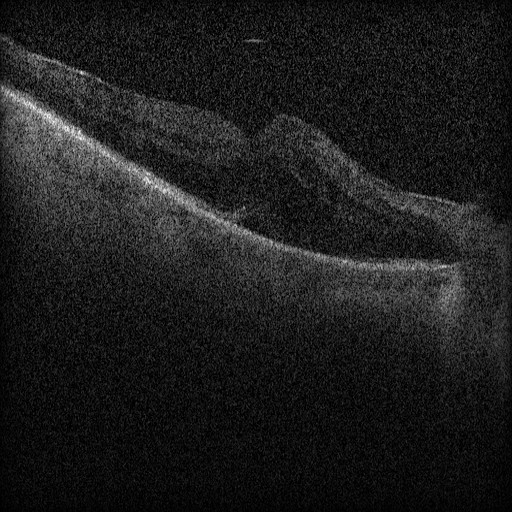
Heidelberg Spectralis; optical coherence tomography scan; SD-OCT; centered on the fovea — Diabetic macular edema (DME).